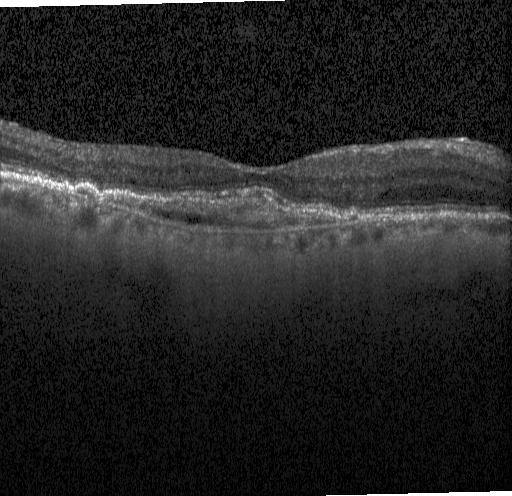
Retinal OCT cross-section showing choroidal neovascularization.